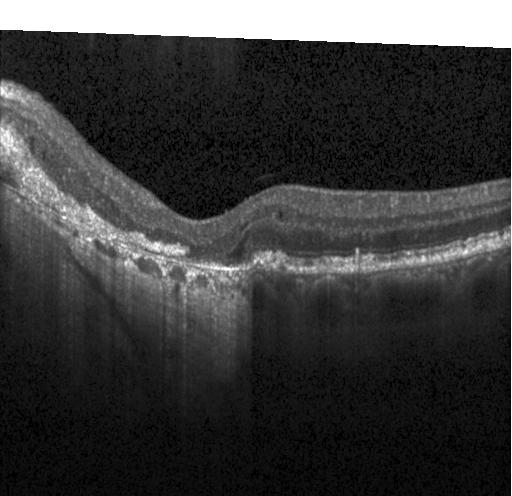
Spectral-domain OCT · macular scan · retinal OCT B-scan.
Diagnosis: a choroidal neovascular membrane.